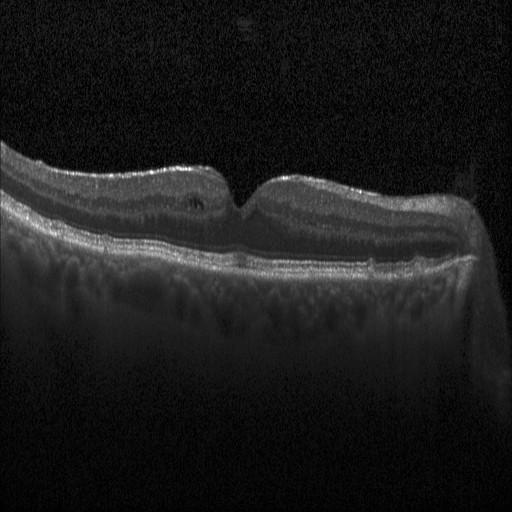 Diagnosis: diabetic macular edema (DME).